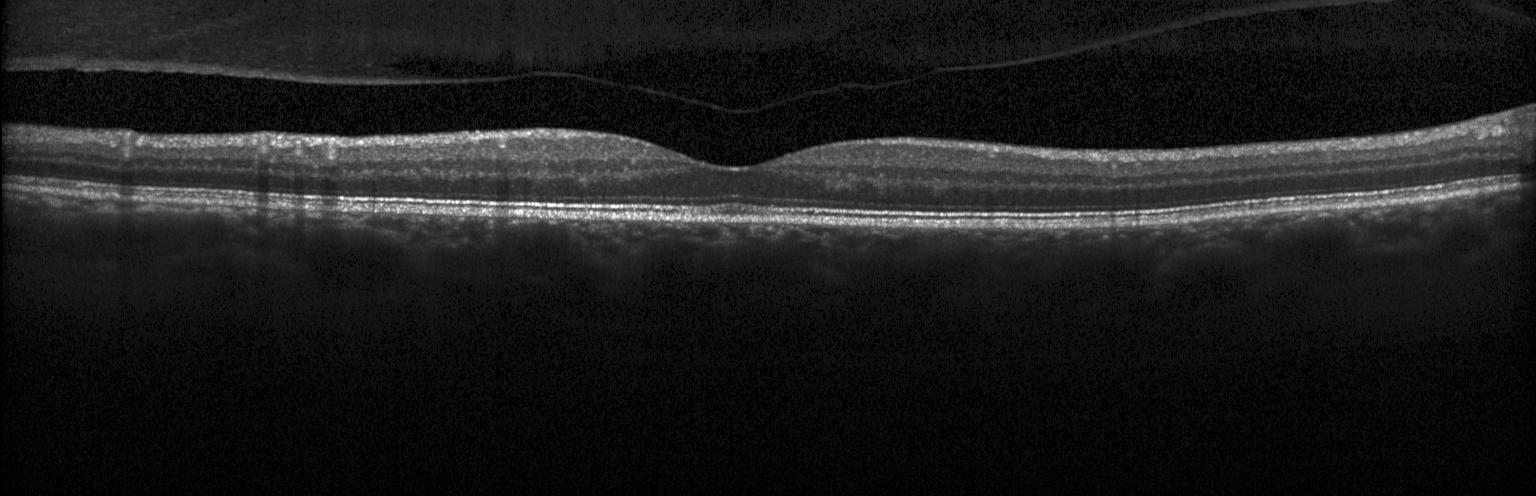 OCT finding: neither CNV, DME, nor drusen.